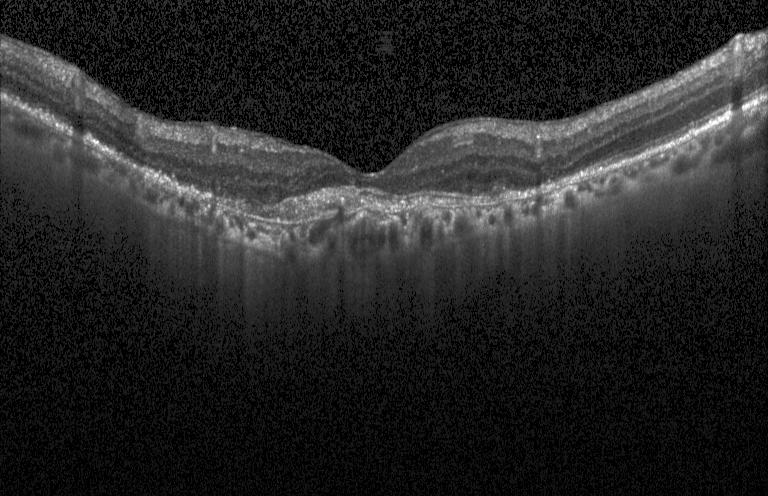 SD-OCT · retinal OCT B-scan · macular scan · acquired on a Heidelberg Spectralis. Diagnosis: a choroidal neovascular membrane.